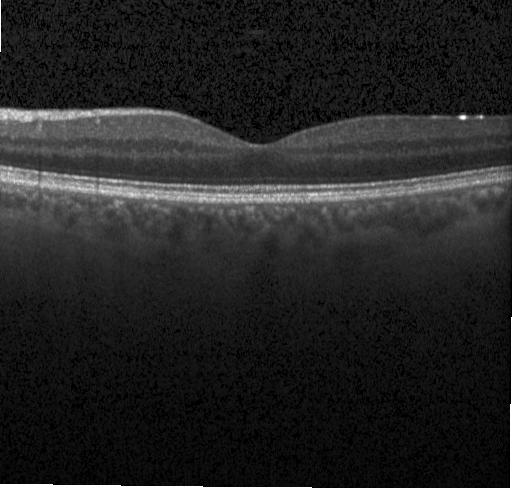
The scan shows no CNV, DME, or drusen.